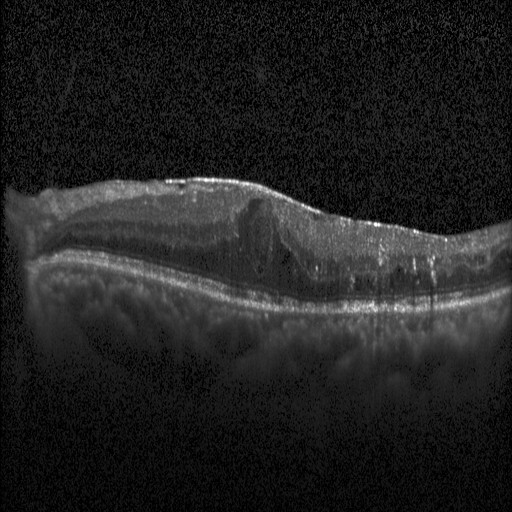
Heidelberg Spectralis. SD-OCT. Horizontal scan through the fovea. OCT B-scan.
The scan shows diabetic macular edema (DME).